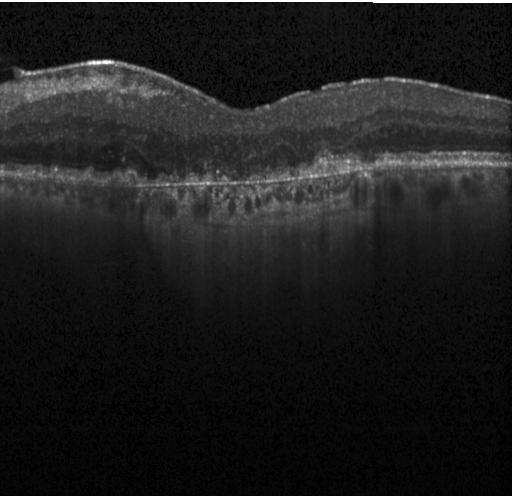 Heidelberg Spectralis, fovea-centered, SD-OCT, OCT line scan. Finding: a choroidal neovascular membrane.